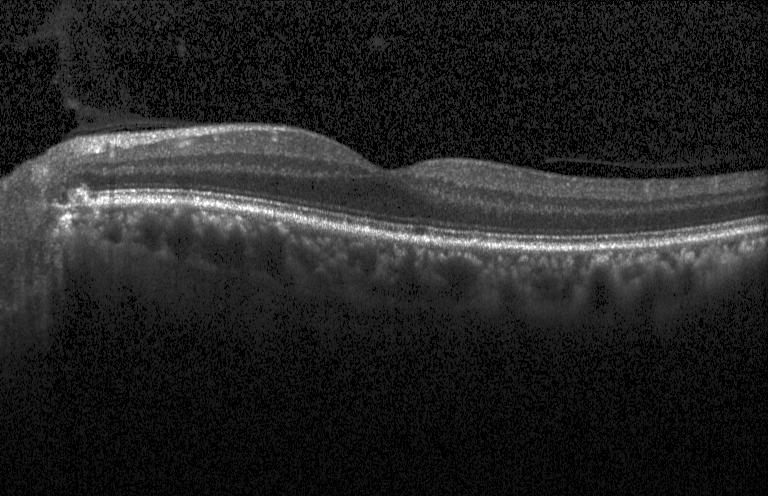
OCT B-scan — OCT finding: no CNV, DME, or drusen.